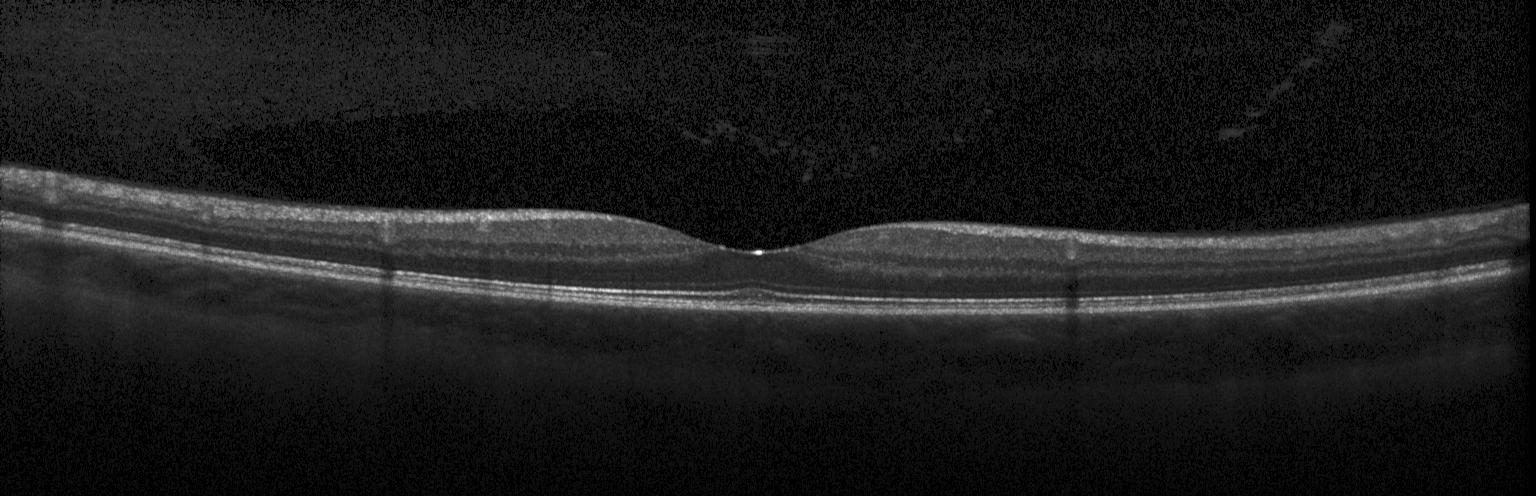 OCT B-scan — Macular OCT: no choroidal neovascularization, diabetic macular edema, or drusen.